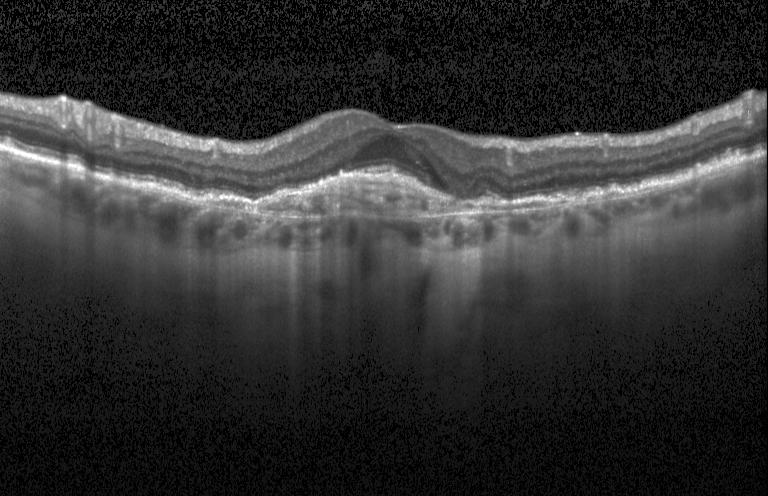

Optical coherence tomography scan; instrument: Heidelberg Spectralis; spectral-domain optical coherence tomography; fovea-centered — Macular OCT: choroidal neovascularization (CNV).